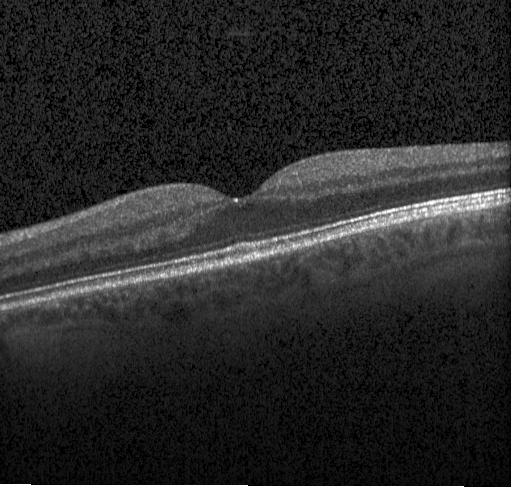
Spectral-domain optical coherence tomography, retinal OCT cross-section
This B-scan demonstrates no choroidal neovascularization, diabetic macular edema, or drusen.